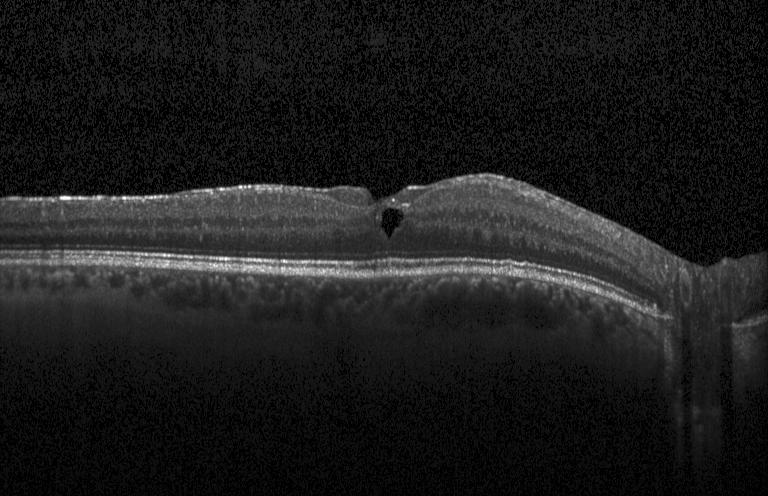
Acquired on a Heidelberg Spectralis; optical coherence tomography scan.
Assessment: DME.